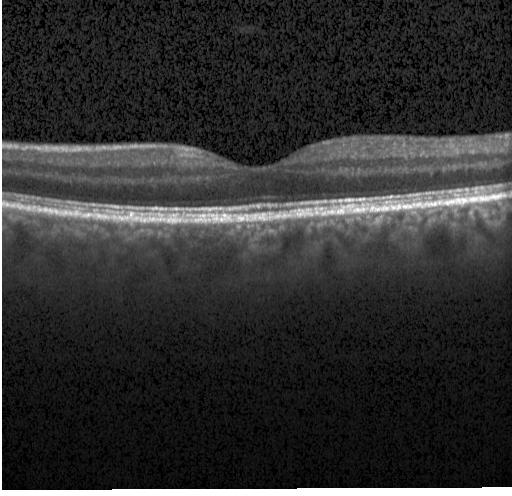 Impression: neither choroidal neovascularization, diabetic macular edema, nor drusen.